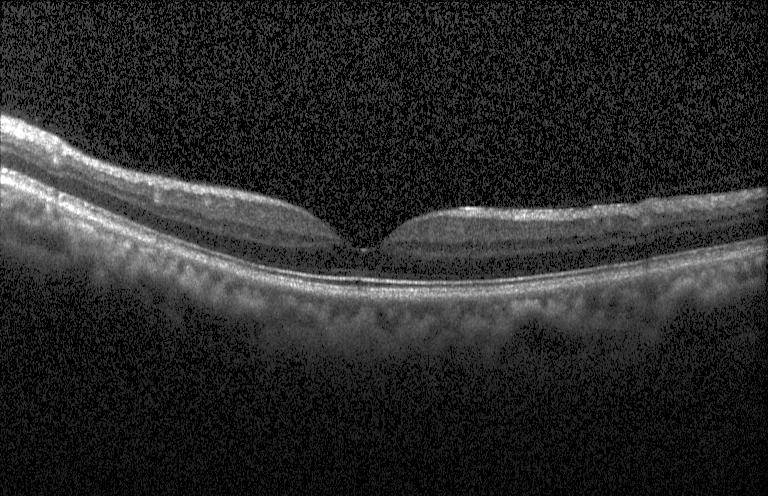

Instrument: Heidelberg Spectralis; OCT B-scan — No choroidal neovascularization, no diabetic macular edema, and no drusen.